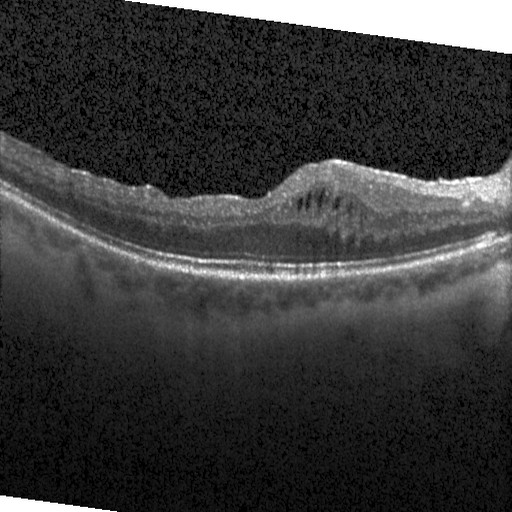

Impression: diabetic macular edema.